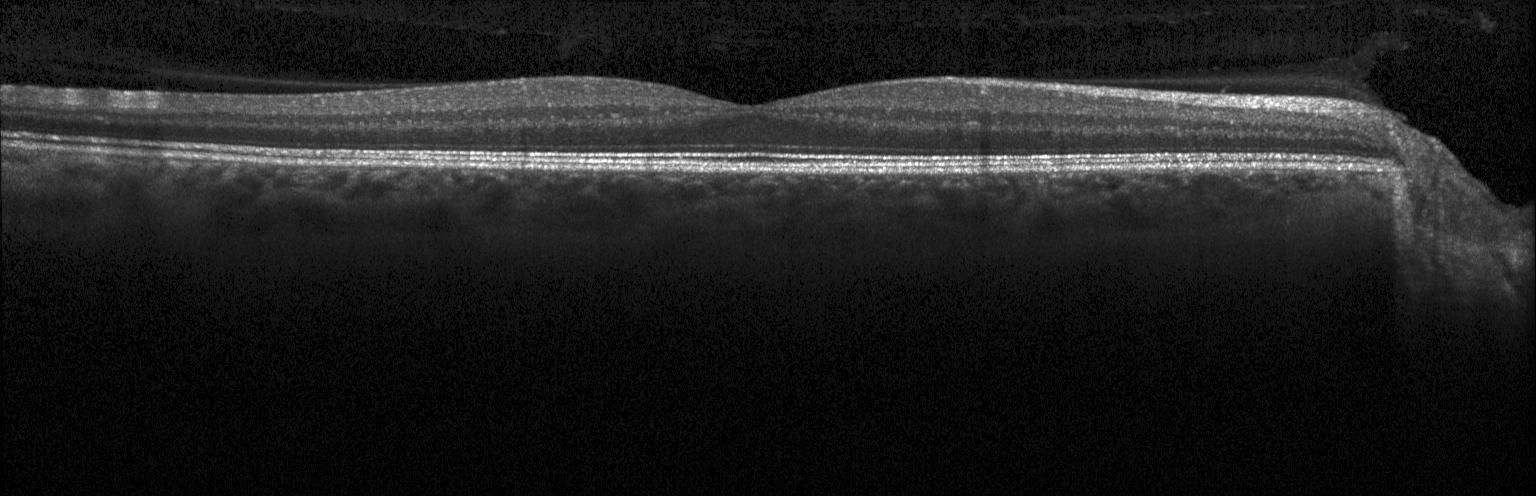

Instrument: Heidelberg Spectralis, centered on the fovea, spectral-domain OCT, retinal OCT B-scan. Diagnosis: no choroidal neovascularization, diabetic macular edema, or drusen.